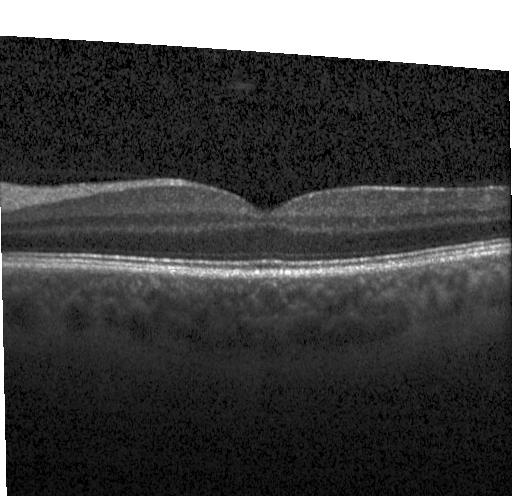 Macular OCT demonstrating no CNV, DME, or drusen.